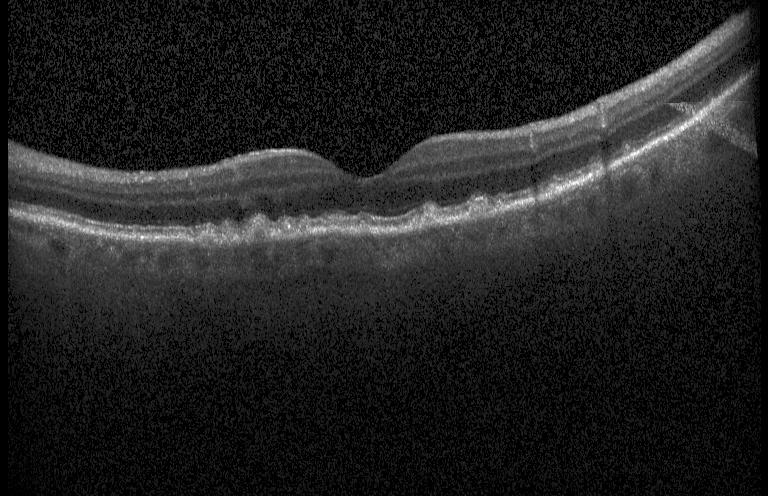 Heidelberg Spectralis OCT system · fovea-centered · spectral-domain optical coherence tomography · OCT B-scan — Diagnosis: drusen.